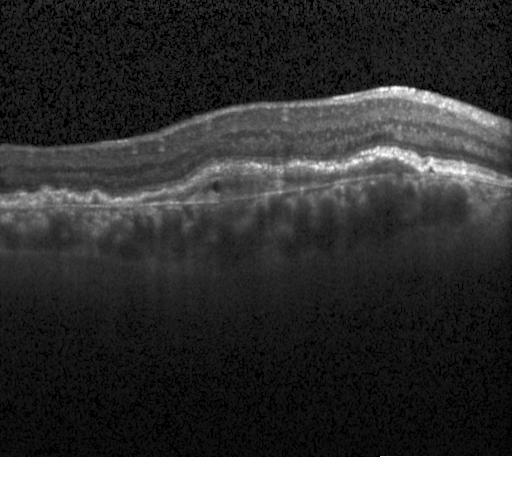
Optical coherence tomography scan
Choroidal neovascularization.